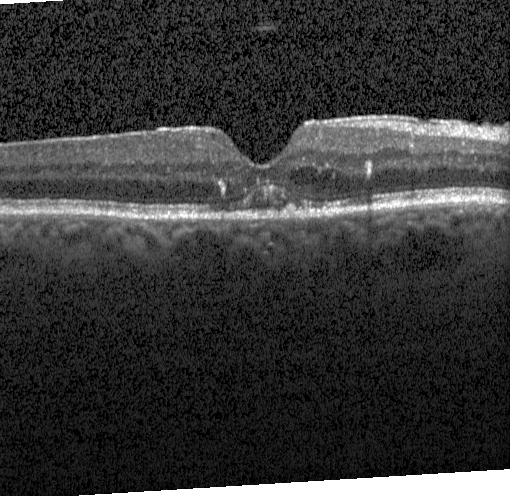

The scan shows choroidal neovascularization (CNV).